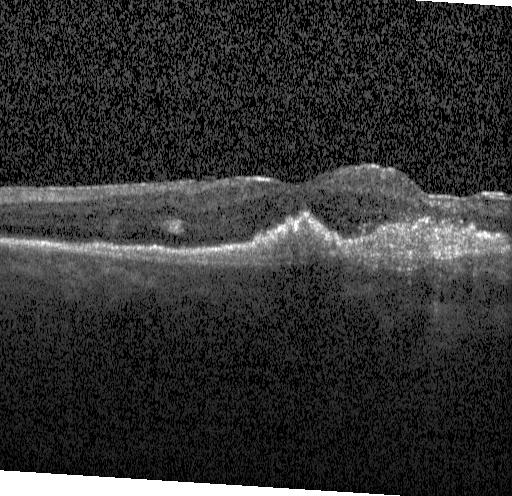

Optical coherence tomography B-scan. Dx: choroidal neovascularization (CNV).